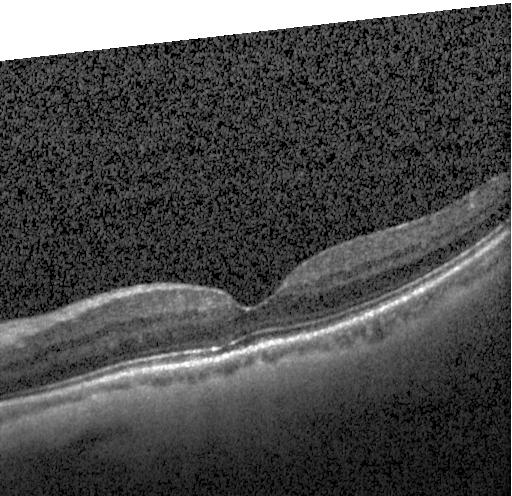
Diagnosis: no evidence of choroidal neovascularization, diabetic macular edema, or drusen.